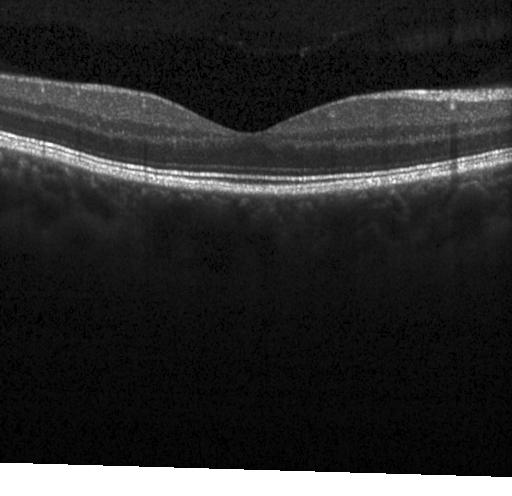 Centered on the fovea; Heidelberg Spectralis; retinal OCT cross-section; spectral-domain optical coherence tomography
This B-scan demonstrates no CNV, no DME, and no drusen.